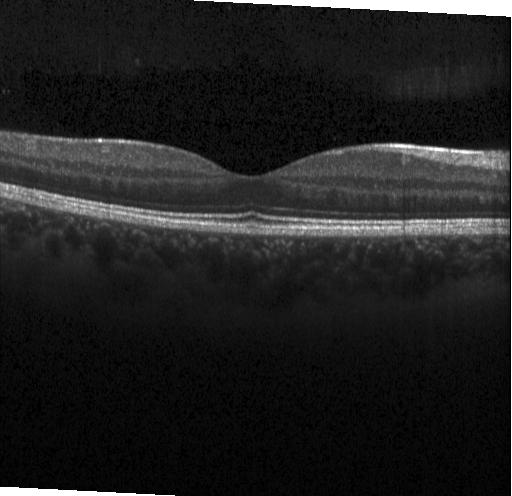
OCT scan showing neither choroidal neovascularization, diabetic macular edema, nor drusen.